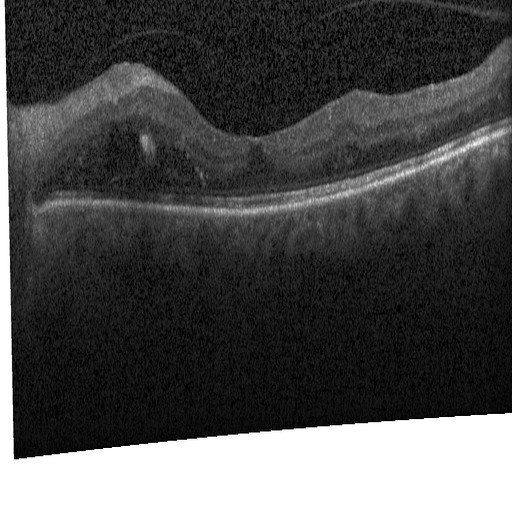
Impression: diabetic macular edema (DME).